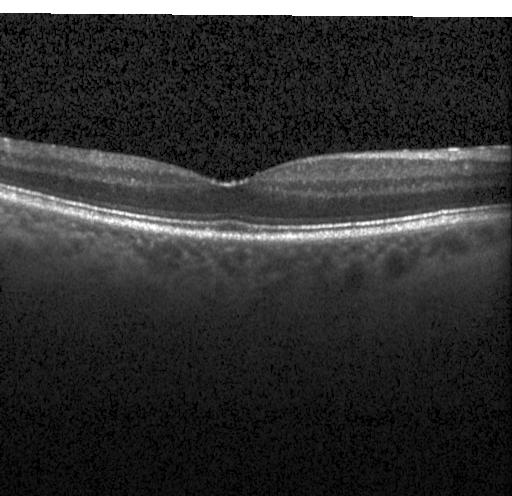 Diagnosis: no choroidal neovascularization, diabetic macular edema, or drusen.